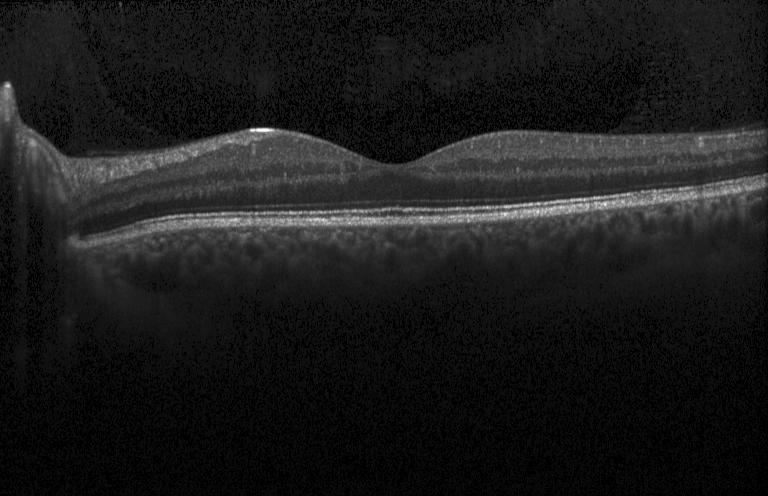

Retinal OCT B-scan
OCT finding: no CNV, no DME, and no drusen.